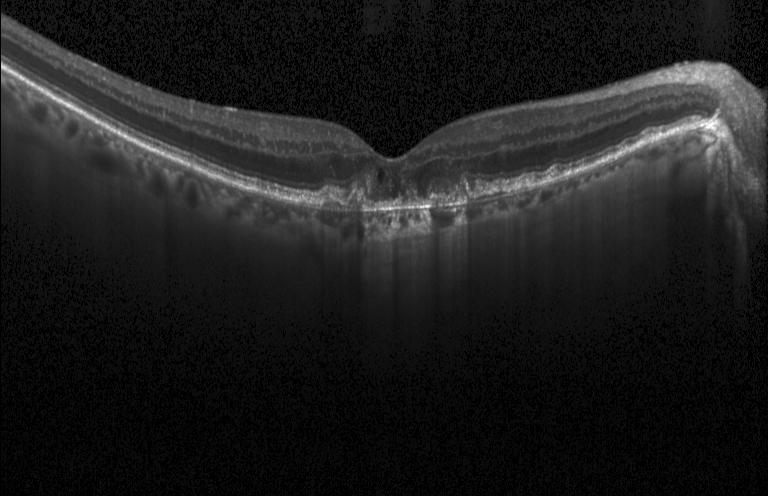
OCT finding: a choroidal neovascular membrane.